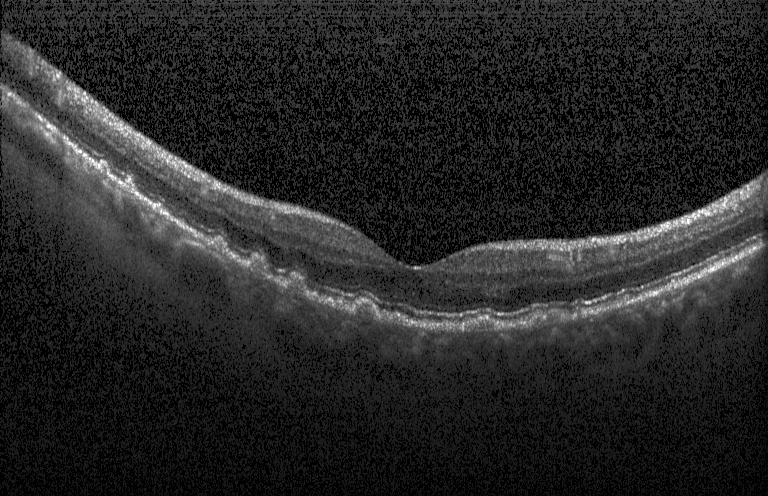
Assessment: drusen.